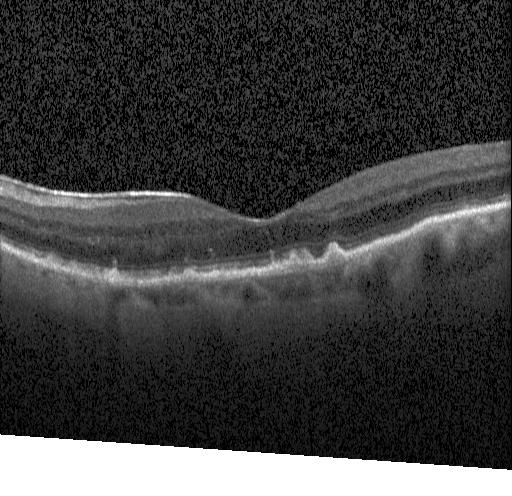 Macular OCT: sub-RPE drusenoid deposits.